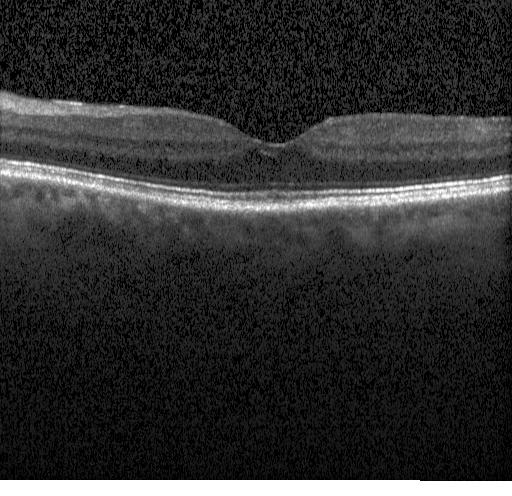

SD-OCT · OCT B-scan — The scan shows no evidence of choroidal neovascularization, diabetic macular edema, or drusen.